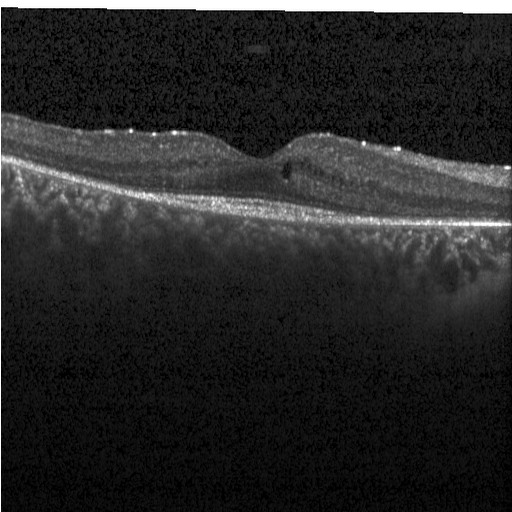

Spectral-domain OCT B-scan: diabetic macular edema.